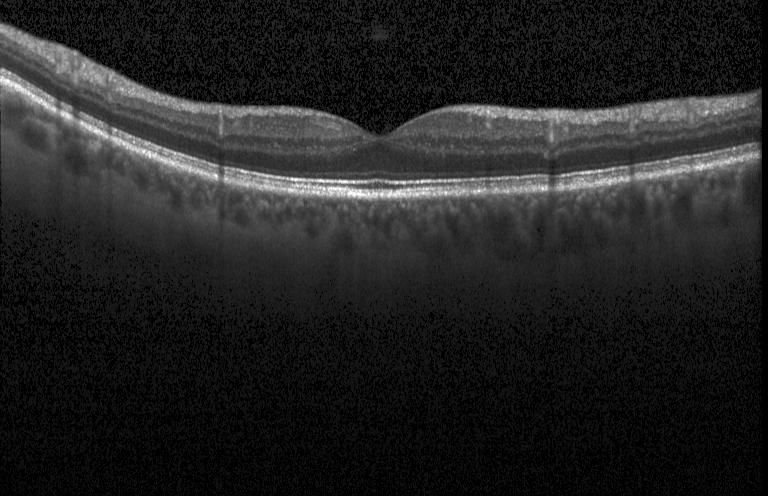 Spectral-domain OCT, through the macula, OCT line scan — Neither choroidal neovascularization, diabetic macular edema, nor drusen.